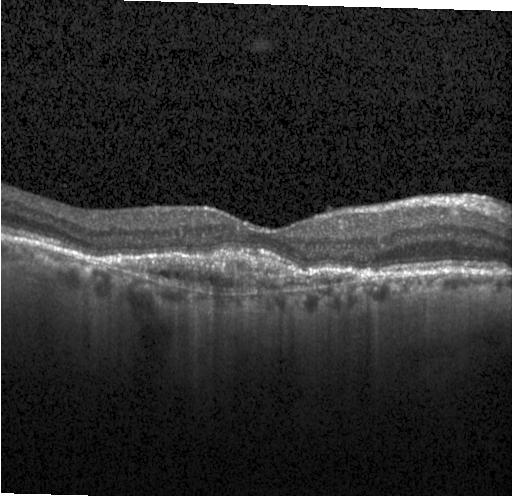

Retinal OCT B-scan · centered on the fovea — Impression: CNV.